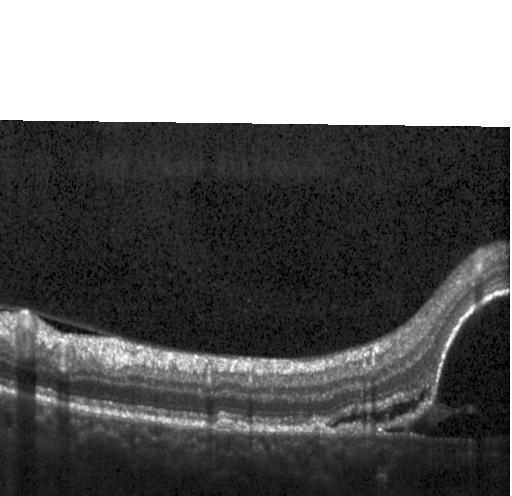 Finding: a choroidal neovascular membrane.